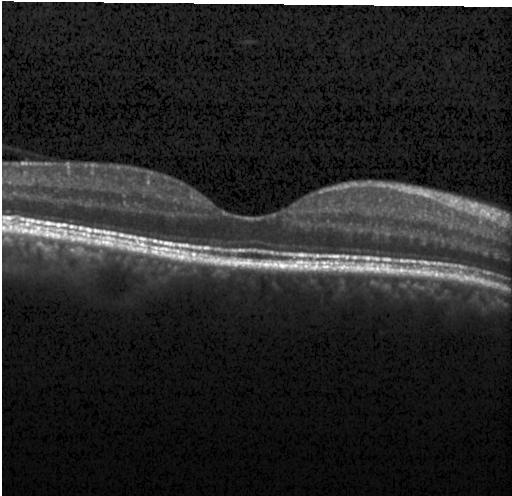
Retinal OCT B-scan. Centered on the fovea. Impression: no CNV, no DME, and no drusen.